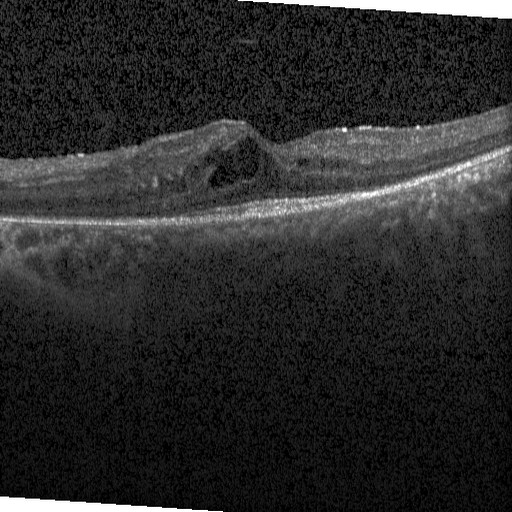
Heidelberg Spectralis, spectral-domain optical coherence tomography, optical coherence tomography scan. The scan shows DME.